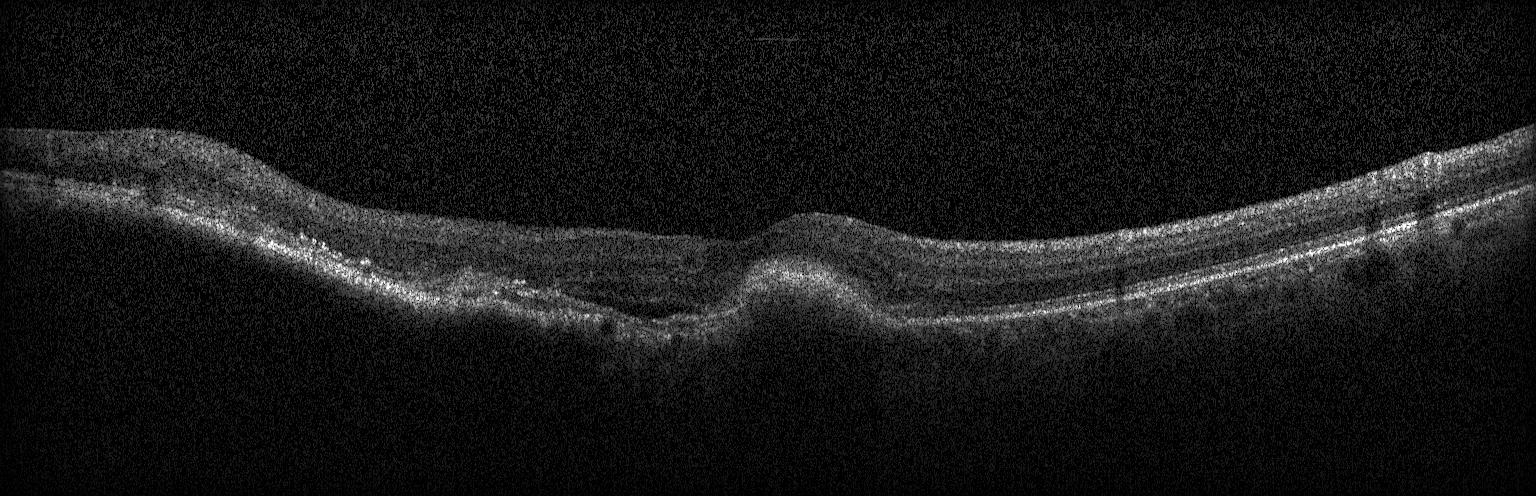 Fovea-centered. Retinal OCT B-scan — This B-scan demonstrates a choroidal neovascular membrane.